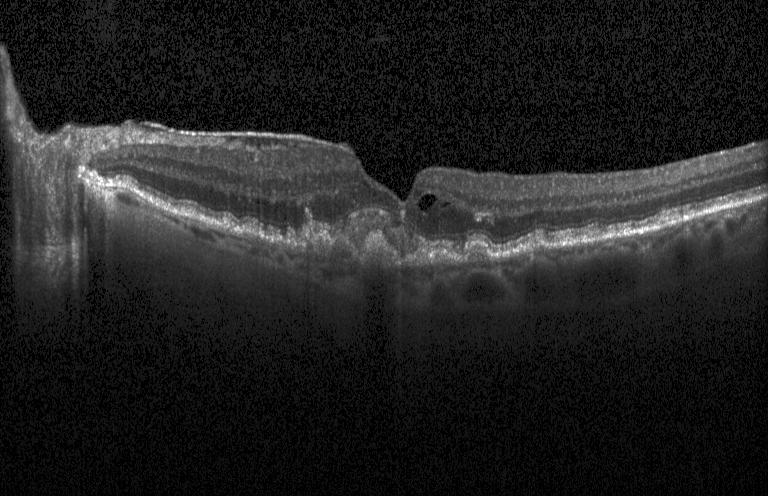
Macular OCT: choroidal neovascularization (CNV).